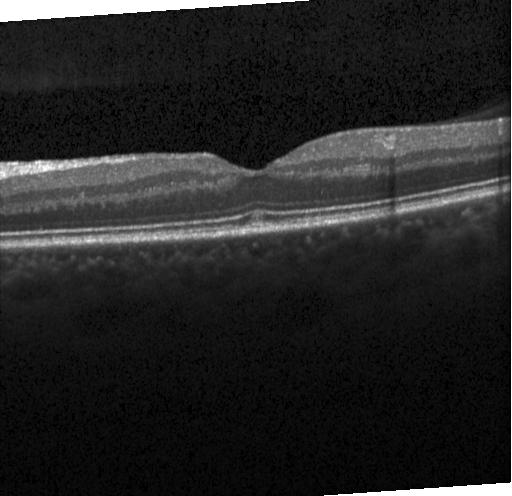 OCT B-scan.
Finding: no evidence of choroidal neovascularization, diabetic macular edema, or drusen.